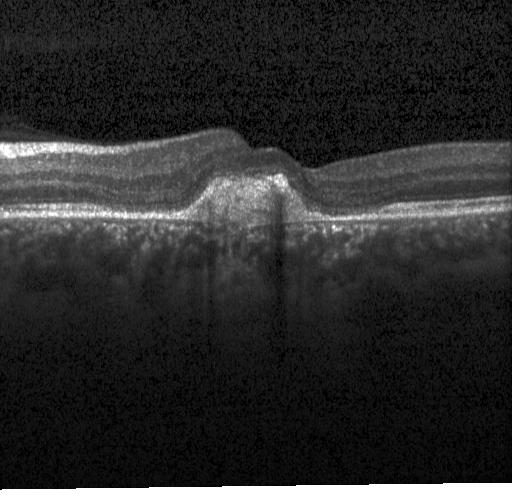
This B-scan demonstrates CNV.